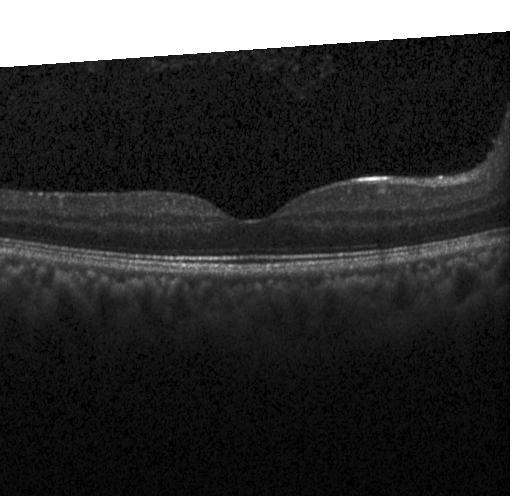

OCT line scan; fovea-centered.
No evidence of CNV, DME, or drusen.